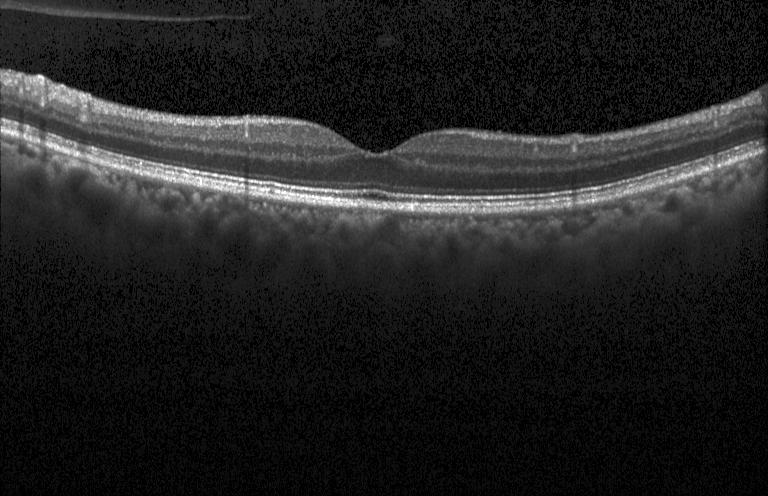
Optical coherence tomography scan; spectral-domain optical coherence tomography; instrument: Heidelberg Spectralis; macular scan
Macular OCT: no evidence of CNV, DME, or drusen.